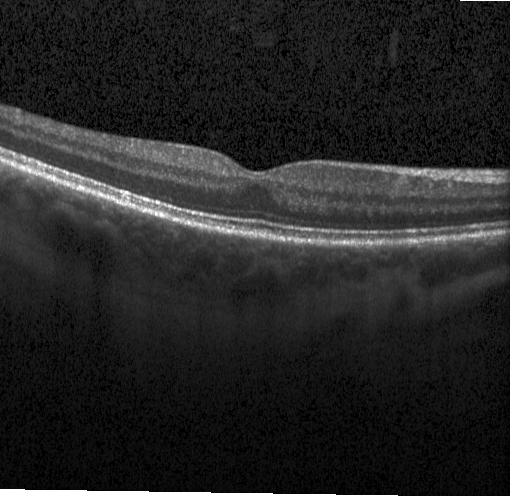
Diagnosis: no evidence of choroidal neovascularization, diabetic macular edema, or drusen.